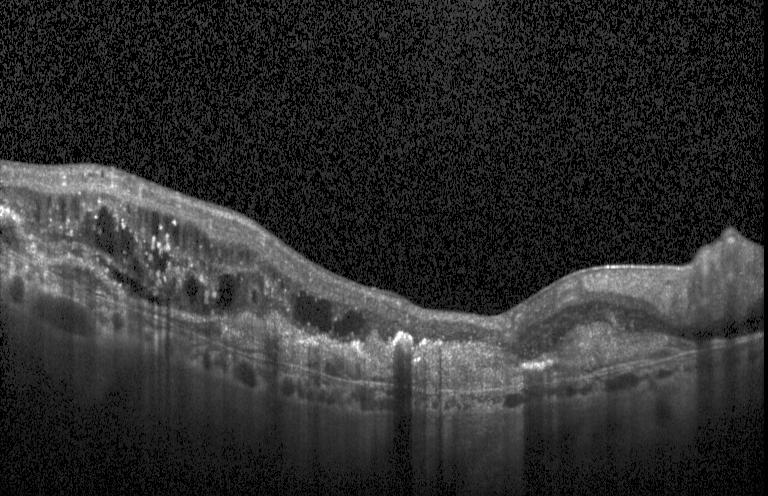 Retinal OCT B-scan.
A choroidal neovascular membrane.